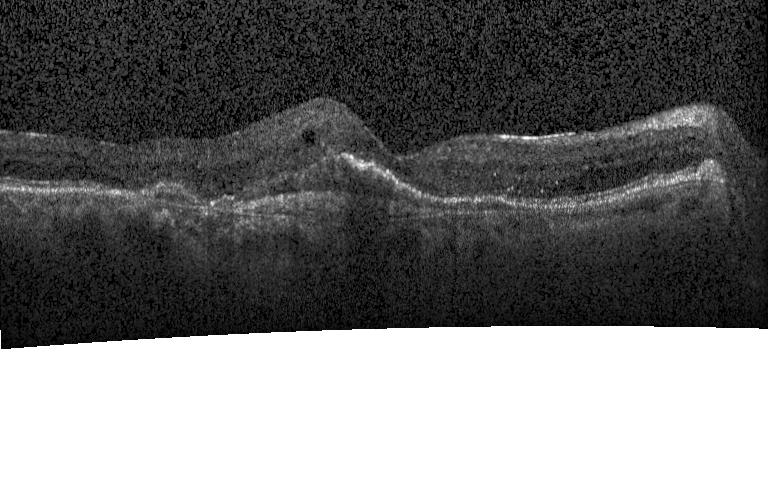

Retinal OCT B-scan.
Impression: a choroidal neovascular membrane.